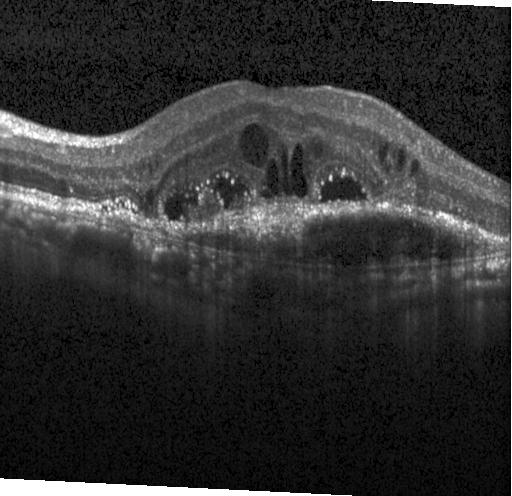 Acquired on a Heidelberg Spectralis, retinal OCT cross-section
This B-scan demonstrates choroidal neovascularization.